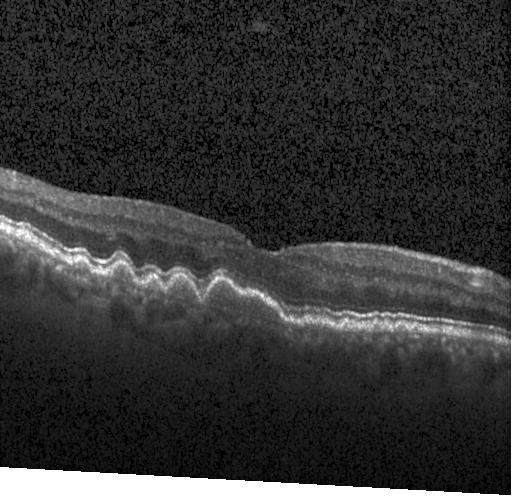

Centered on the fovea, optical coherence tomography B-scan, SD-OCT — Impression: multiple drusen.